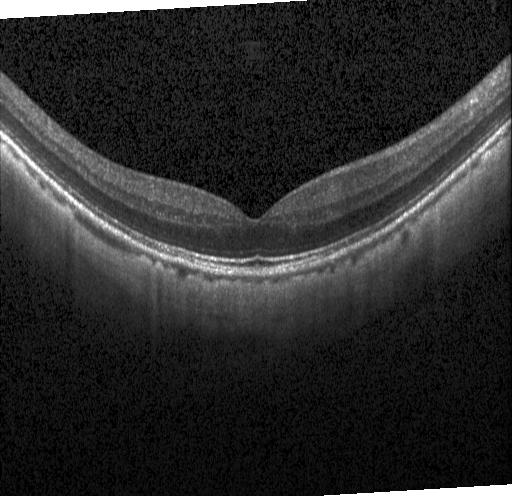

OCT line scan. Instrument: Heidelberg Spectralis. Neither choroidal neovascularization, diabetic macular edema, nor drusen.